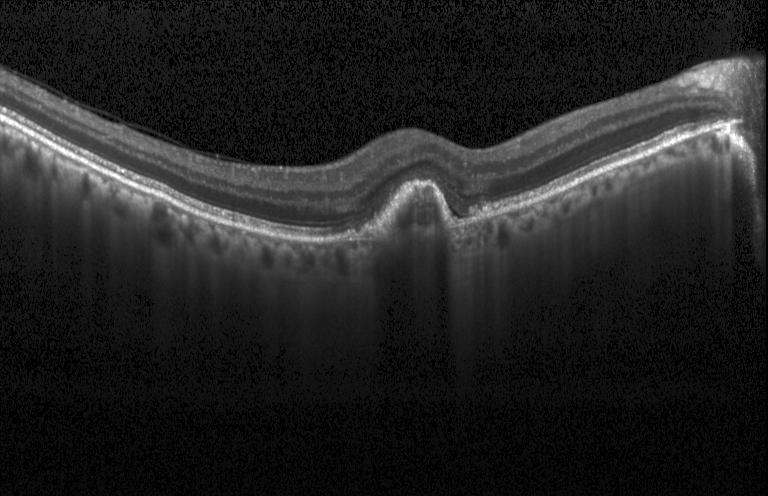 Finding: a choroidal neovascular membrane.